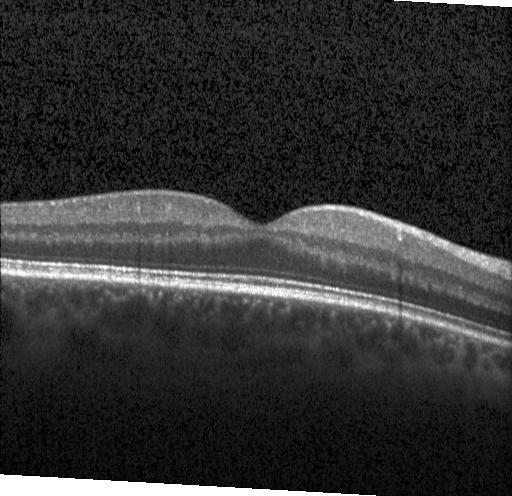

OCT line scan. Instrument: Heidelberg Spectralis
Diagnosis: no CNV, no DME, and no drusen.